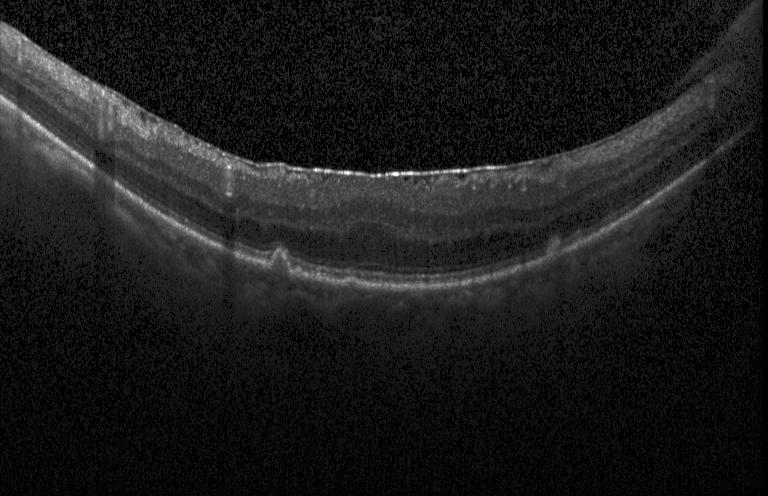 This B-scan demonstrates drusen.